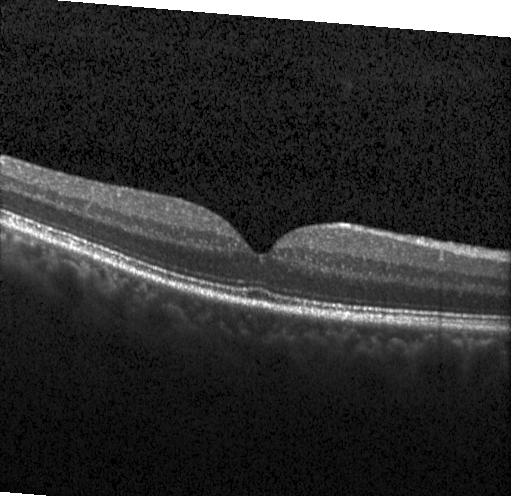 Macular OCT demonstrating neither choroidal neovascularization, diabetic macular edema, nor drusen.